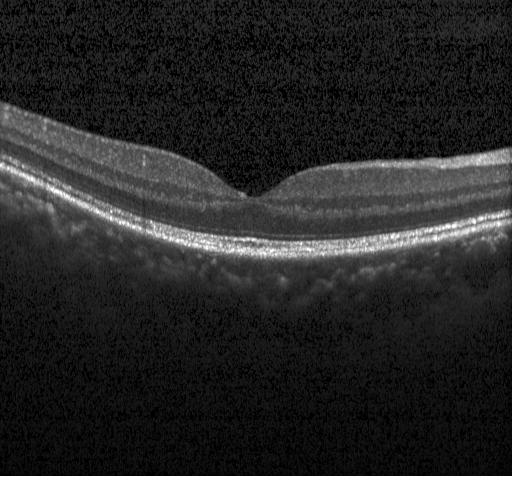 Acquired on a Heidelberg Spectralis; SD-OCT; retinal OCT cross-section.
Macular OCT: neither CNV, DME, nor drusen.